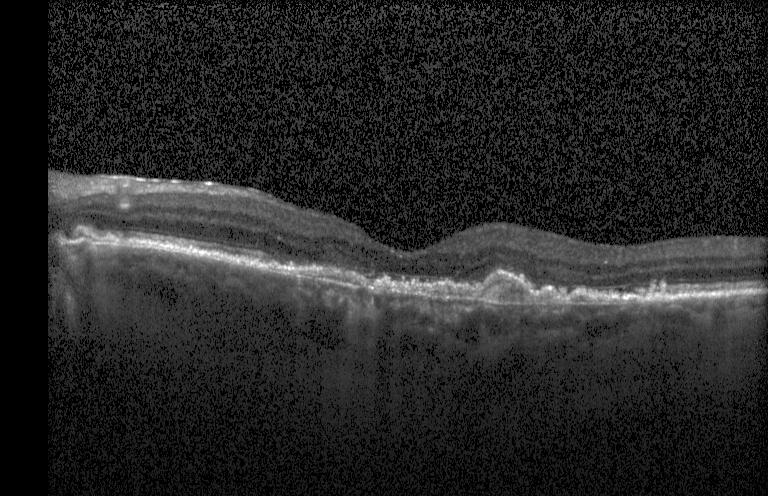 Horizontal scan through the fovea. Optical coherence tomography scan. Impression: a choroidal neovascular membrane.